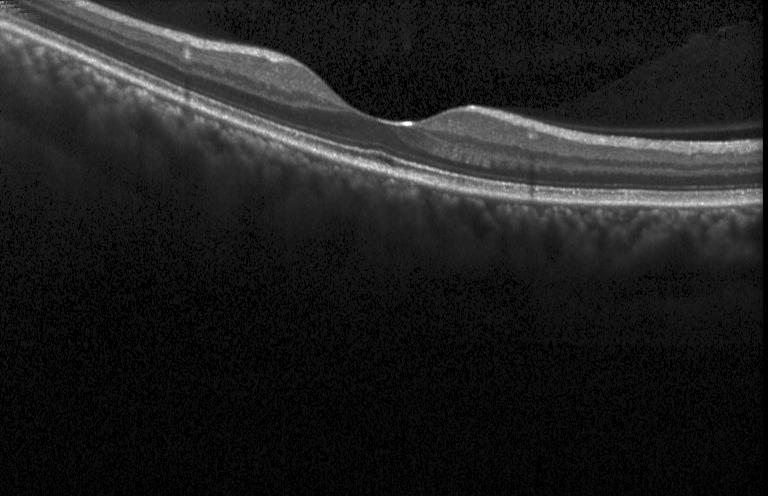 Retinal OCT B-scan; instrument: Heidelberg Spectralis
Impression: no choroidal neovascularization, no diabetic macular edema, and no drusen.